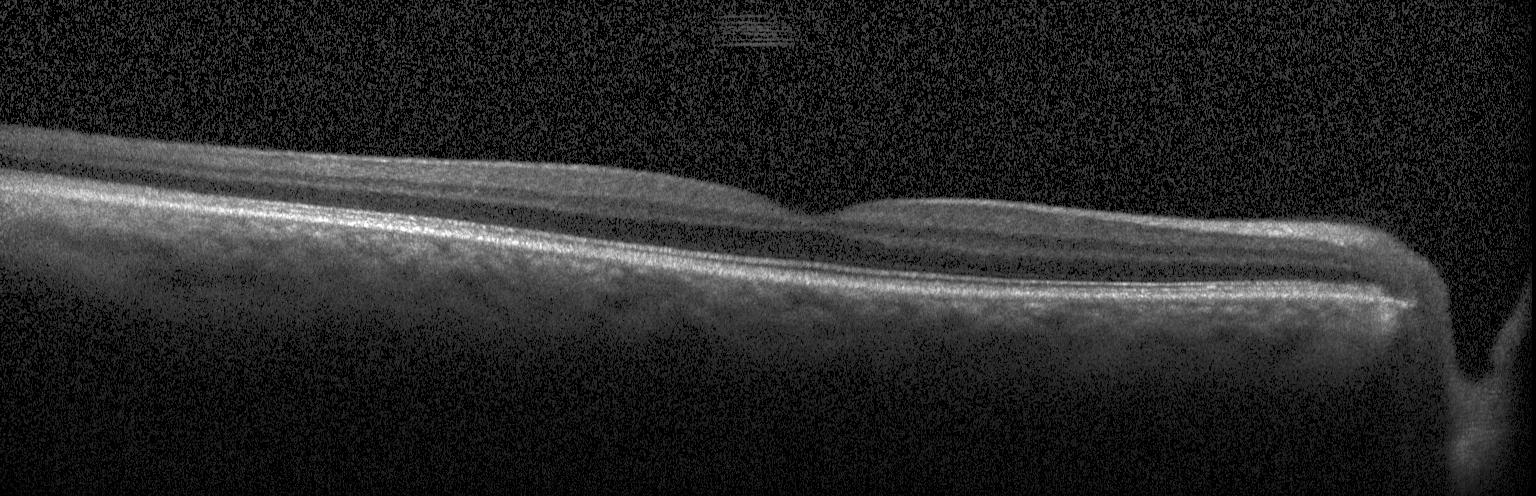 OCT B-scan — Impression: no choroidal neovascularization, diabetic macular edema, or drusen.